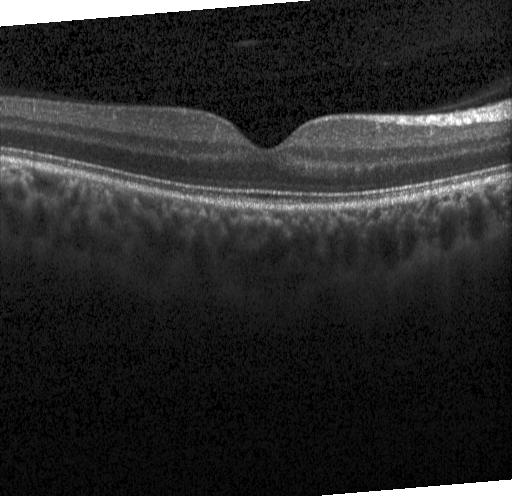

Spectral-domain OCT, OCT B-scan. This B-scan demonstrates no choroidal neovascularization, no diabetic macular edema, and no drusen.